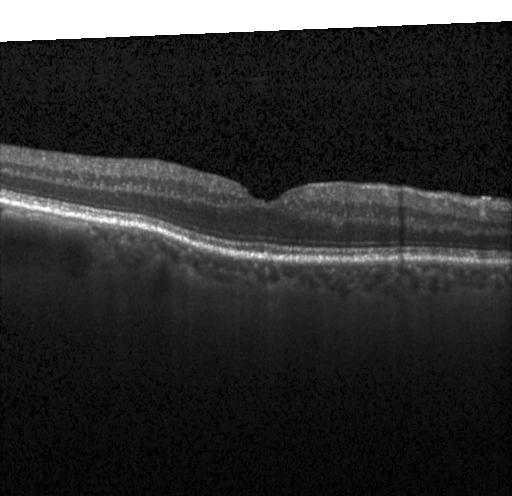
Through the macula; Heidelberg Spectralis OCT system; retinal OCT B-scan; spectral-domain optical coherence tomography
Diagnosis: no choroidal neovascularization, no diabetic macular edema, and no drusen.